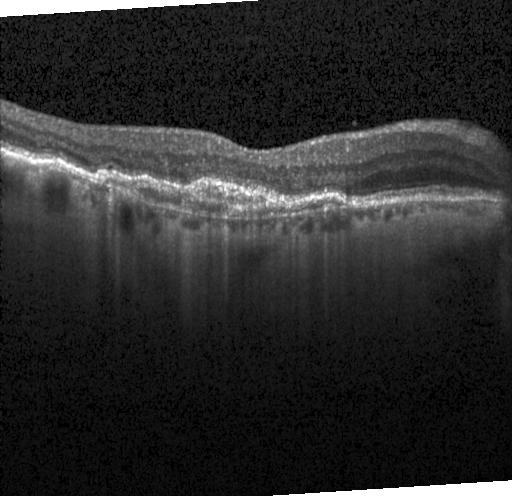 The scan shows choroidal neovascularization (CNV).